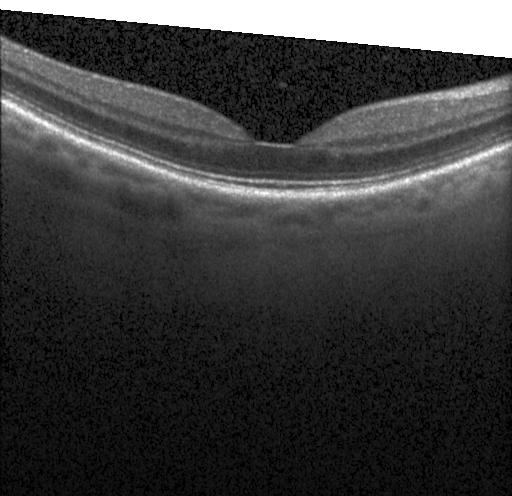 This B-scan demonstrates no evidence of choroidal neovascularization, diabetic macular edema, or drusen.